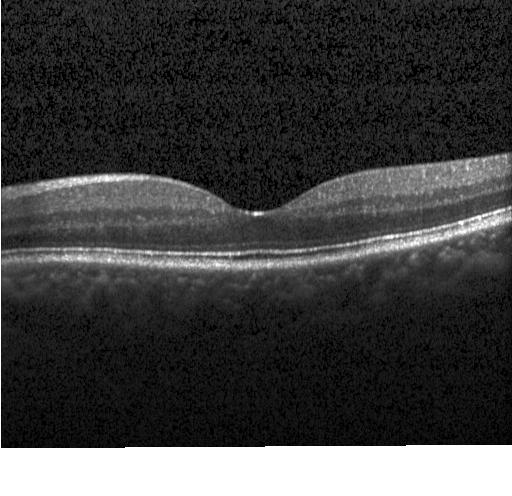 The scan shows no evidence of choroidal neovascularization, diabetic macular edema, or drusen.